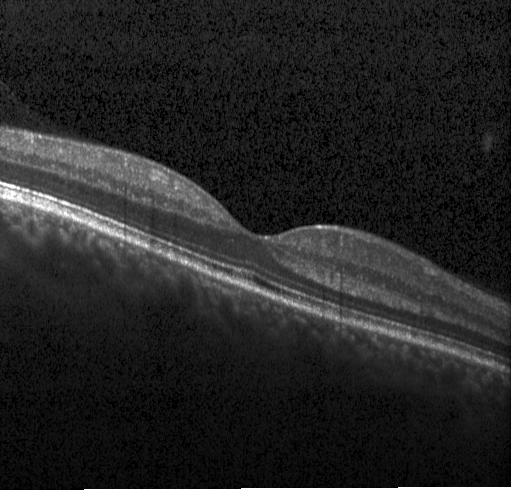

OCT B-scan; centered on the fovea — Assessment: neither choroidal neovascularization, diabetic macular edema, nor drusen.